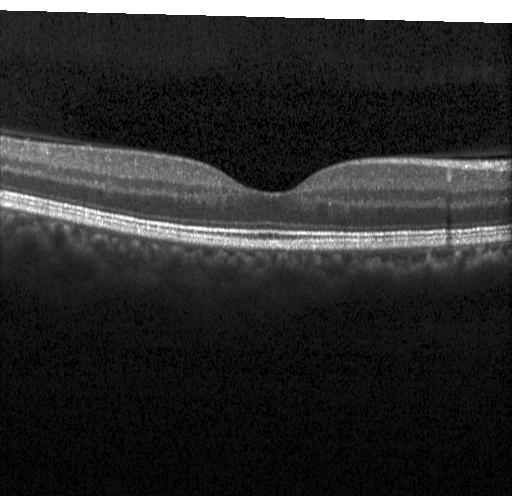

This B-scan demonstrates neither choroidal neovascularization, diabetic macular edema, nor drusen.